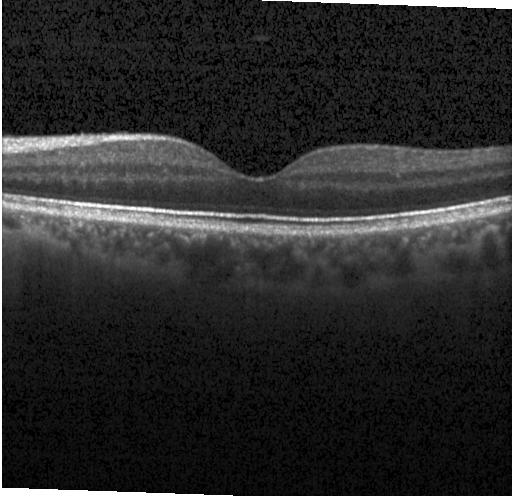 OCT finding: no choroidal neovascularization, diabetic macular edema, or drusen.